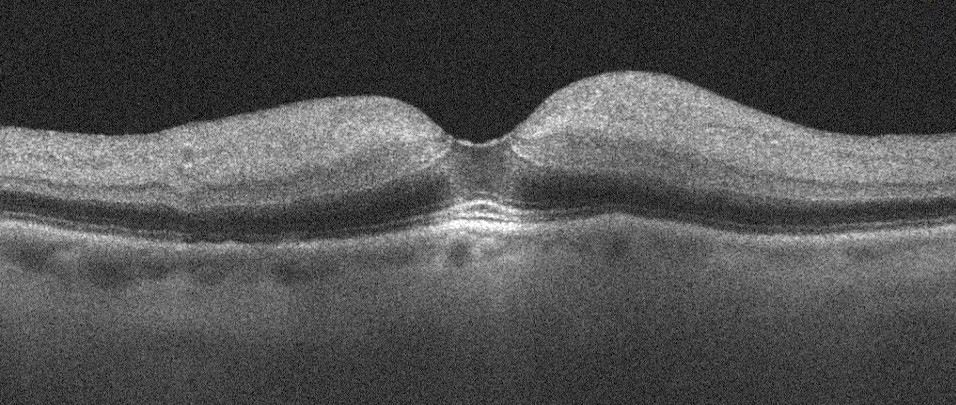
Retinal OCT B-scan
Finding: retinal artery occlusion (RAO).